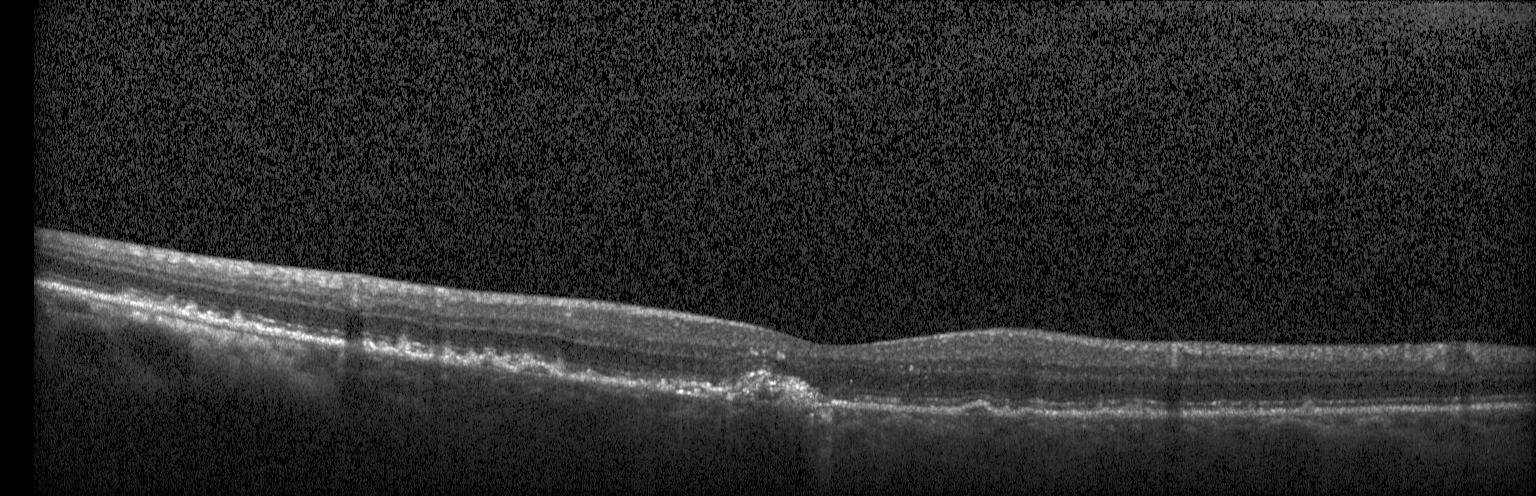 Heidelberg Spectralis. Retinal OCT cross-section. Spectral-domain optical coherence tomography — Impression: a choroidal neovascular membrane.